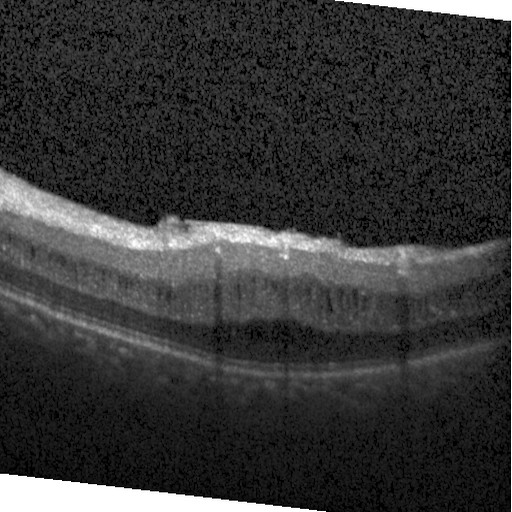

Acquired on a Heidelberg Spectralis. OCT line scan — Finding: diabetic macular edema.